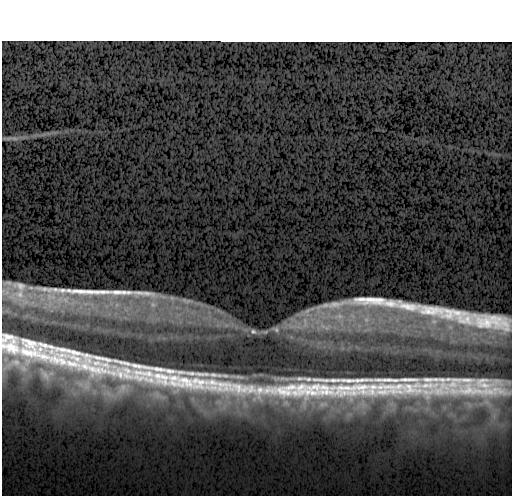
OCT B-scan, spectral-domain optical coherence tomography, instrument: Heidelberg Spectralis.
Finding: no CNV, no DME, and no drusen.